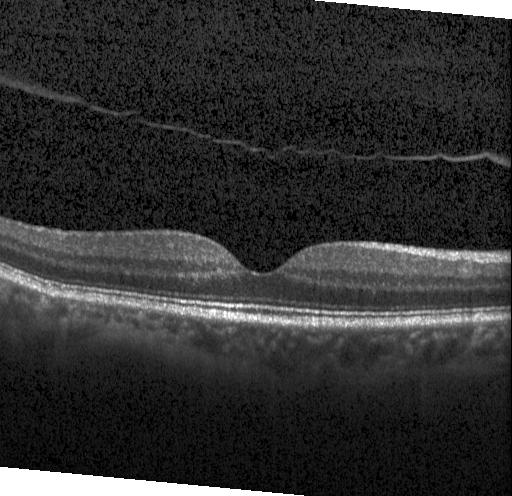

Diagnosis: no evidence of choroidal neovascularization, diabetic macular edema, or drusen.